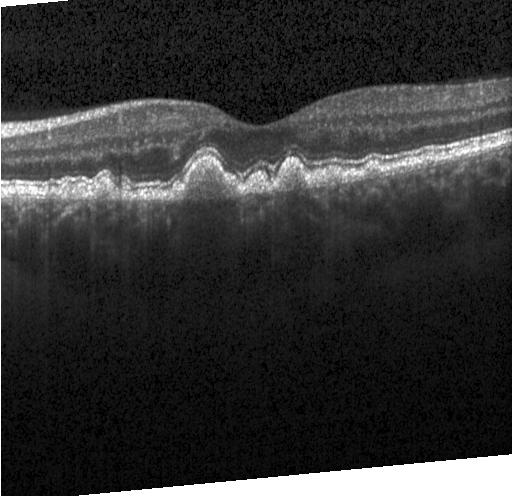

Finding: drusen.